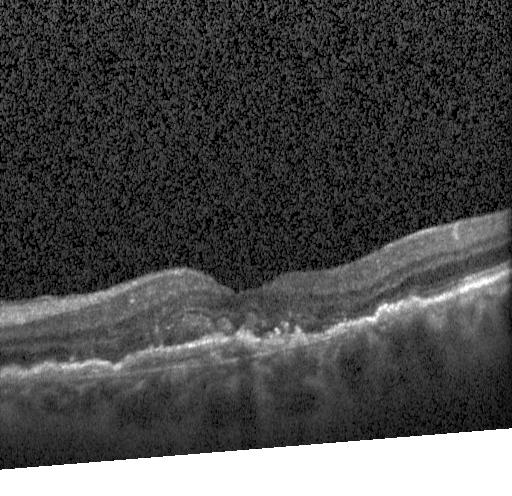 Optical coherence tomography scan
Finding: CNV.